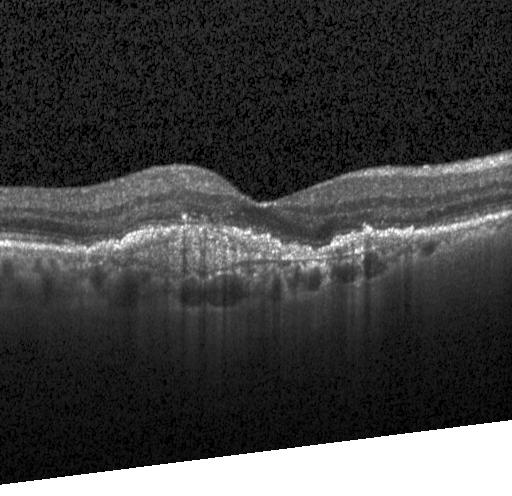

Impression: a choroidal neovascular membrane.